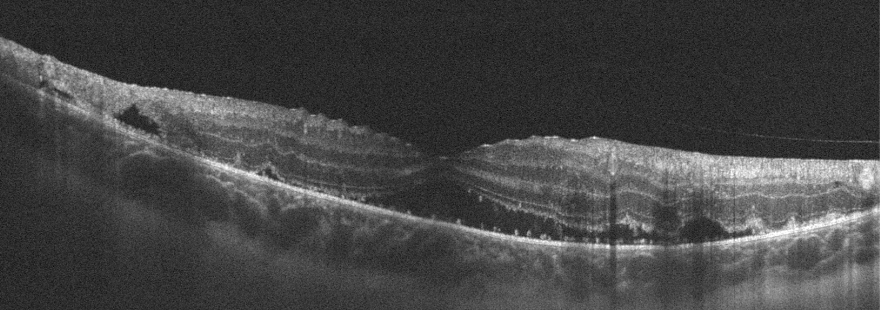
OCT line scan
Assessment: AMD.